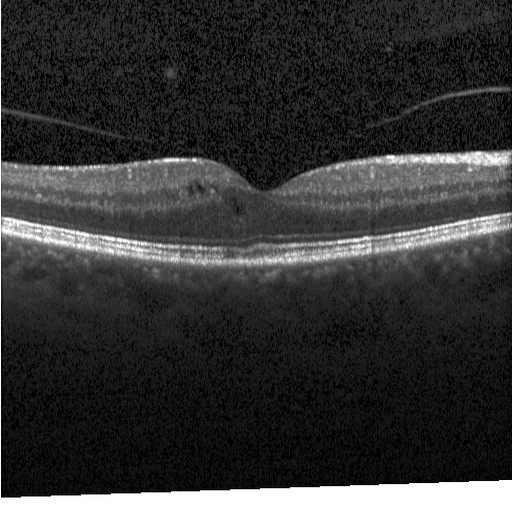

Retinal OCT cross-section showing diabetic macular edema (DME).